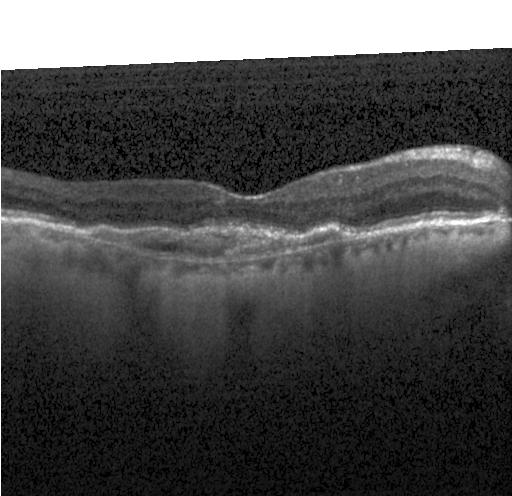

OCT B-scan
Diagnosis: choroidal neovascularization.